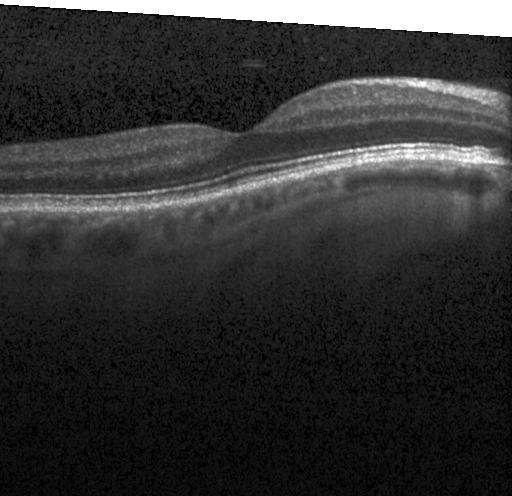
OCT B-scan. Impression: no evidence of choroidal neovascularization, diabetic macular edema, or drusen.